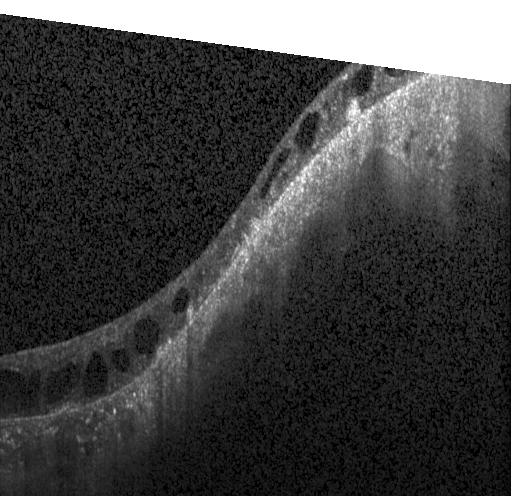

Heidelberg Spectralis OCT system · SD-OCT · OCT line scan. Diabetic macular edema (DME).